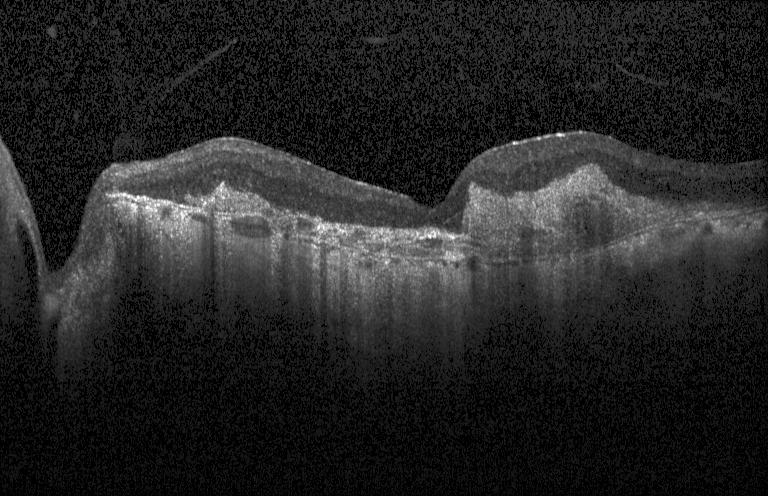

OCT line scan.
Diagnosis: CNV.